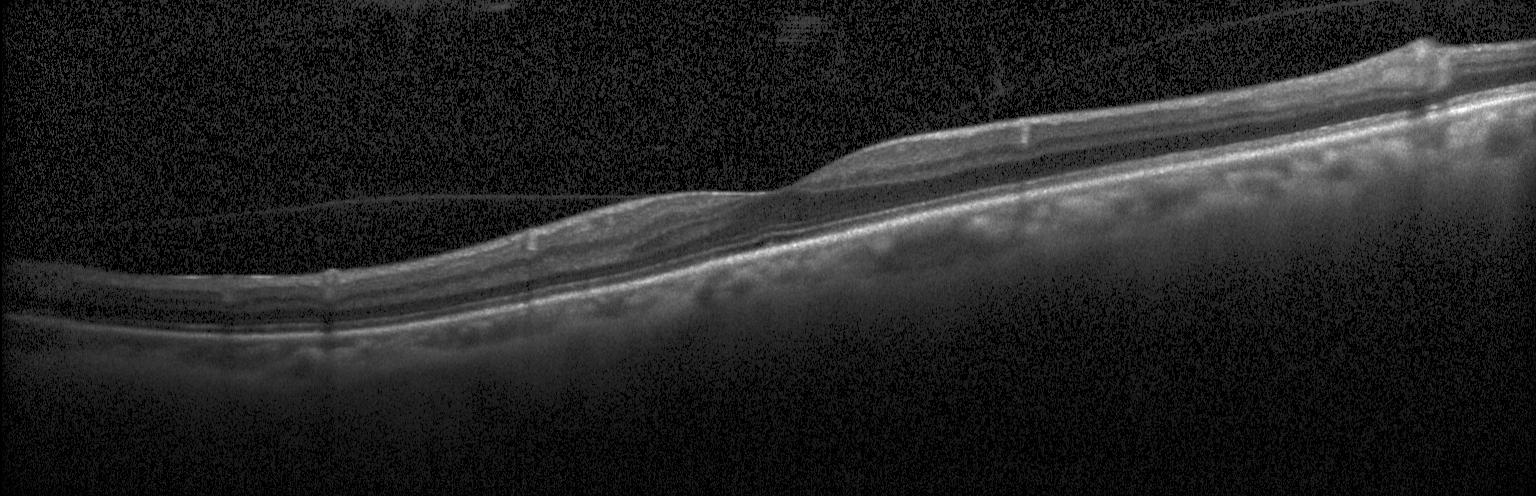

Macular scan · optical coherence tomography scan · spectral-domain OCT. Assessment: no choroidal neovascularization, no diabetic macular edema, and no drusen.